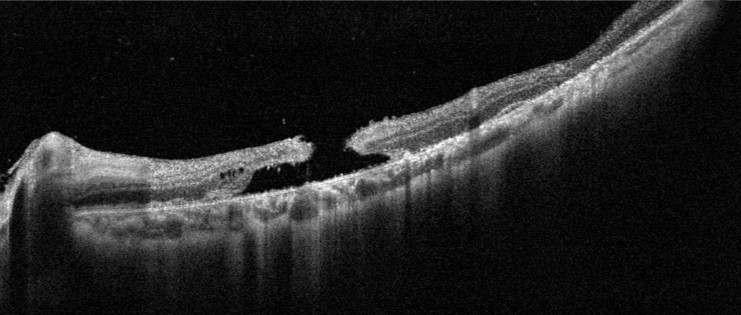

Through the macula · retinal OCT cross-section · acquired on an Optovue Avanti RTVue XR
Finding: vitreomacular interface disease (VID).